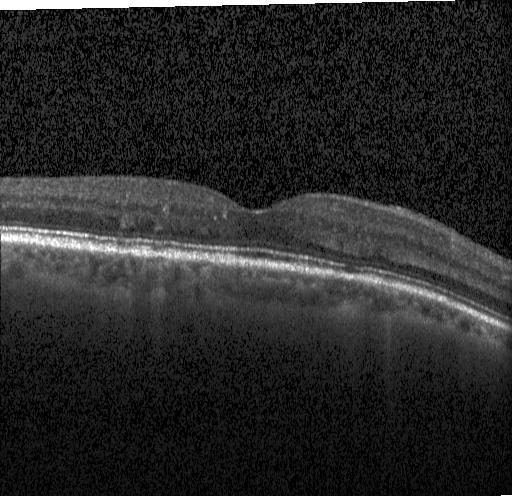

Retinal OCT B-scan — The scan shows DME.